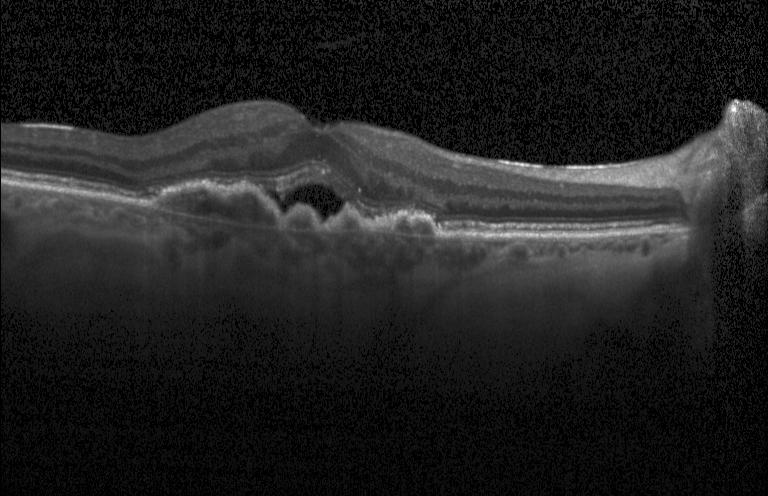
Retinal OCT cross-section; Heidelberg Spectralis OCT system; spectral-domain optical coherence tomography; fovea-centered.
This B-scan demonstrates choroidal neovascularization.